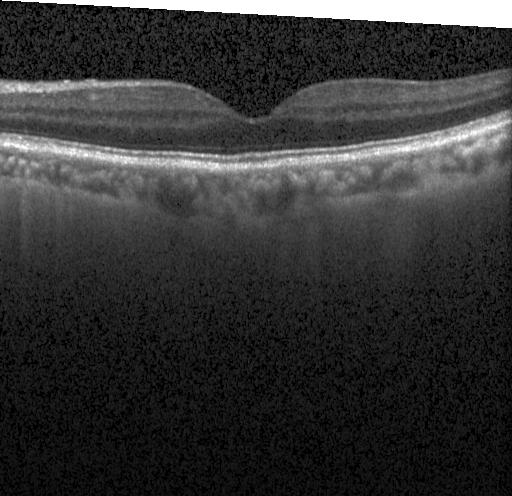
Spectral-domain OCT B-scan: no choroidal neovascularization, no diabetic macular edema, and no drusen.